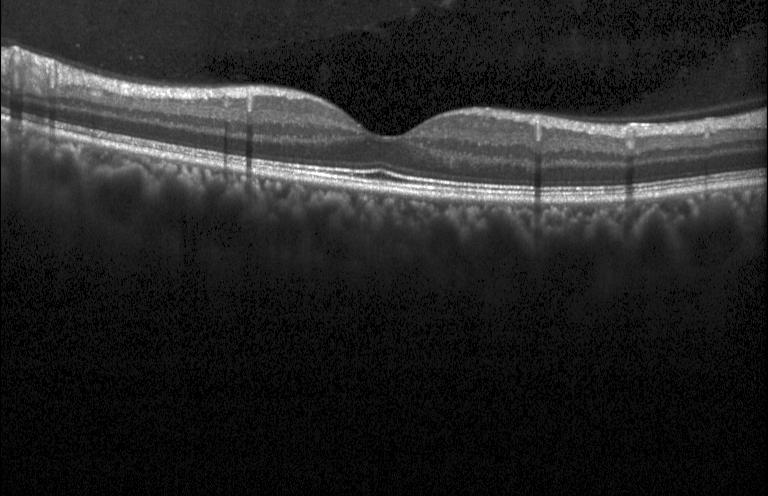 SD-OCT; OCT B-scan
No choroidal neovascularization, no diabetic macular edema, and no drusen.